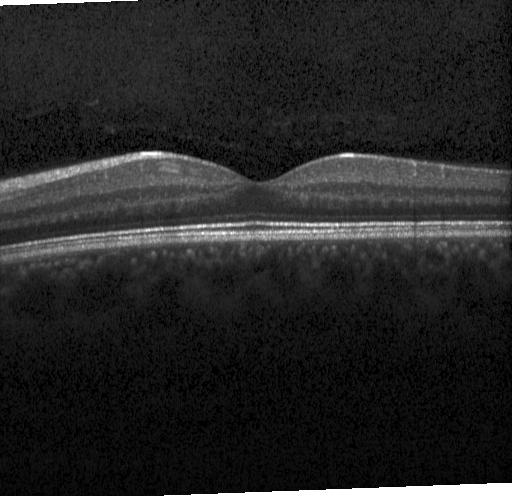
Optical coherence tomography B-scan · spectral-domain optical coherence tomography — Finding: no CNV, no DME, and no drusen.